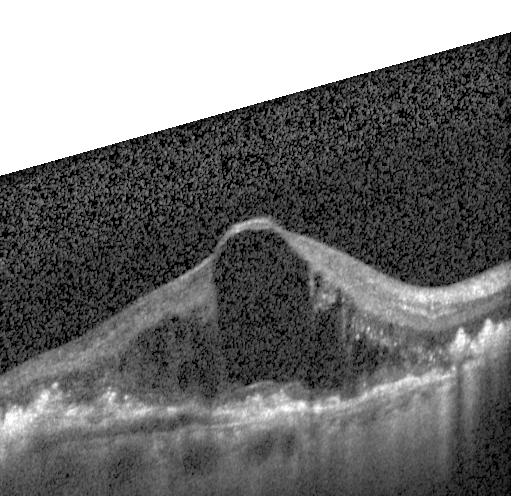

Spectral-domain OCT, acquired on a Heidelberg Spectralis, horizontal scan through the fovea, retinal OCT B-scan.
Finding: a choroidal neovascular membrane.